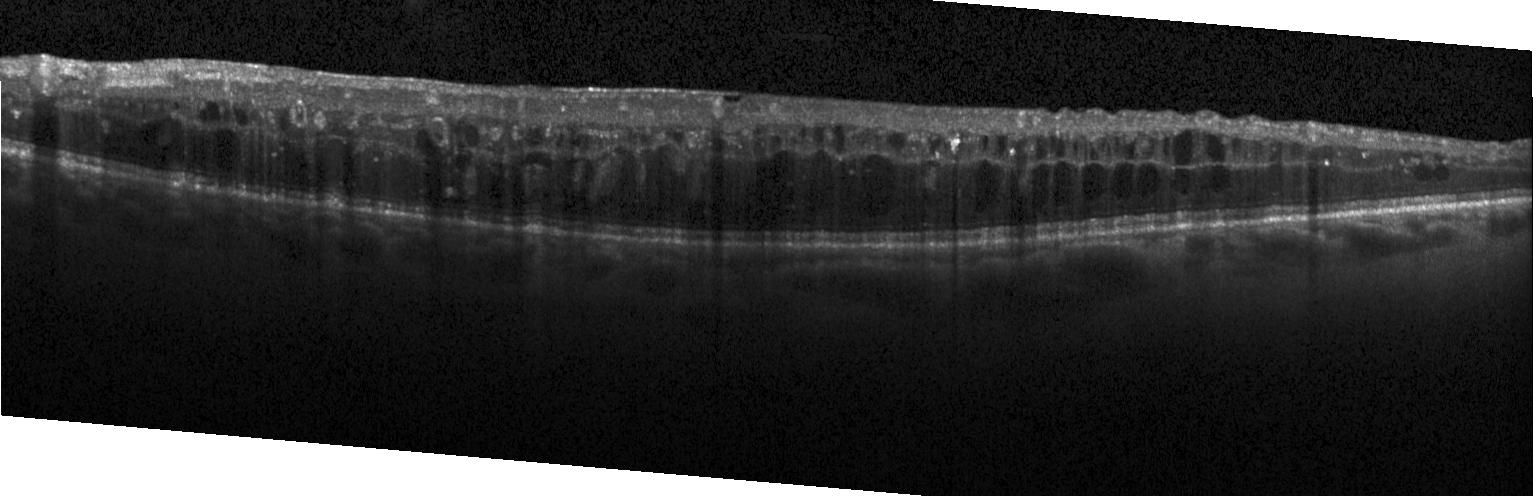 OCT B-scan
Impression: DME.